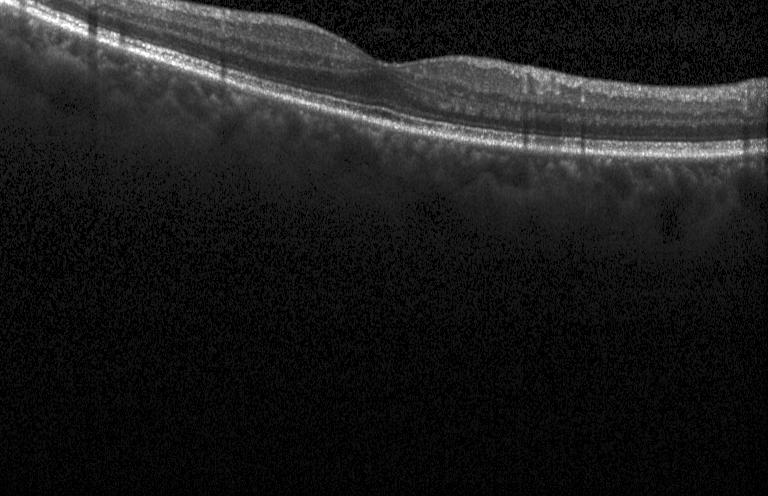

Retinal OCT cross-section.
Impression: neither choroidal neovascularization, diabetic macular edema, nor drusen.